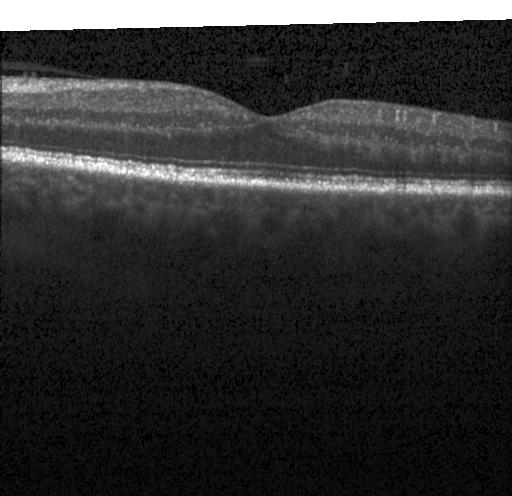

Impression: no CNV, no DME, and no drusen.